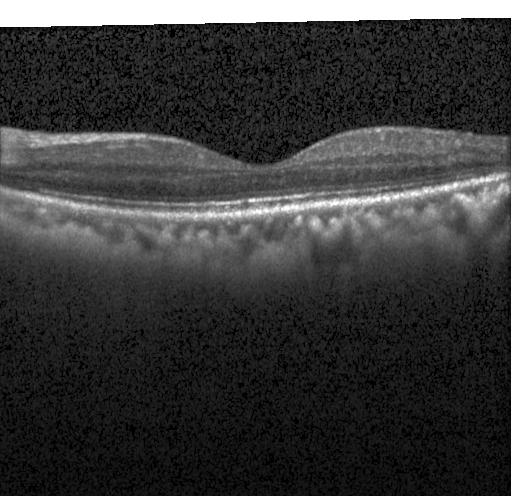 OCT line scan; through the macula; Heidelberg Spectralis; spectral-domain optical coherence tomography — No choroidal neovascularization, diabetic macular edema, or drusen.